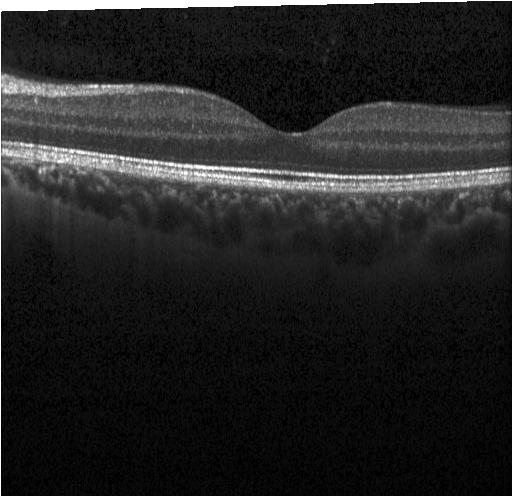
Retinal OCT cross-section showing no evidence of CNV, DME, or drusen.